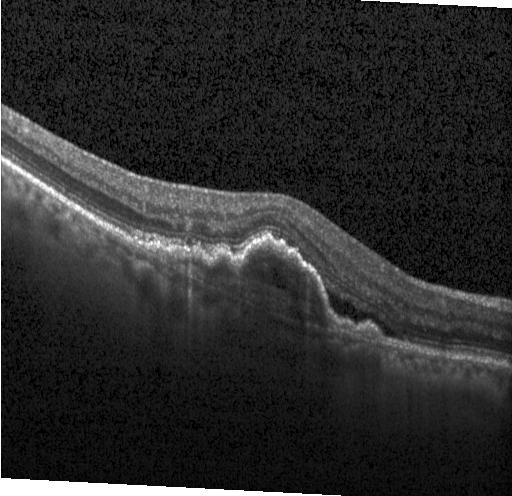

Spectral-domain OCT · retinal OCT cross-section · horizontal scan through the fovea. Finding: a choroidal neovascular membrane.